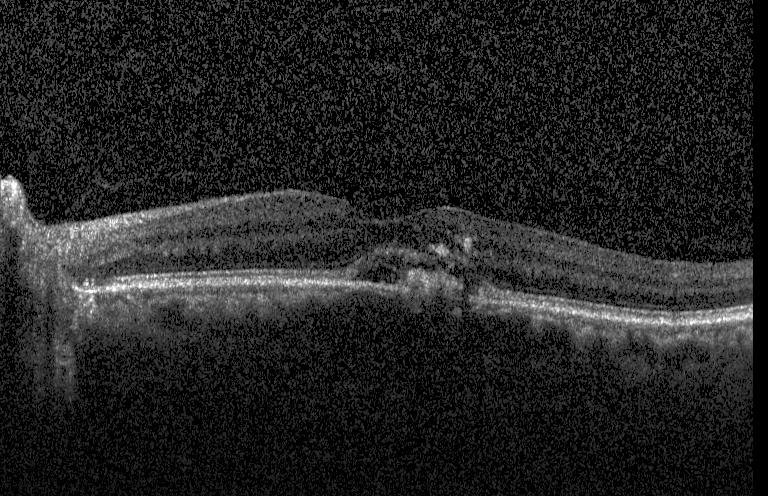
Spectral-domain optical coherence tomography; retinal OCT cross-section; macular scan; instrument: Heidelberg Spectralis
Assessment: a choroidal neovascular membrane.